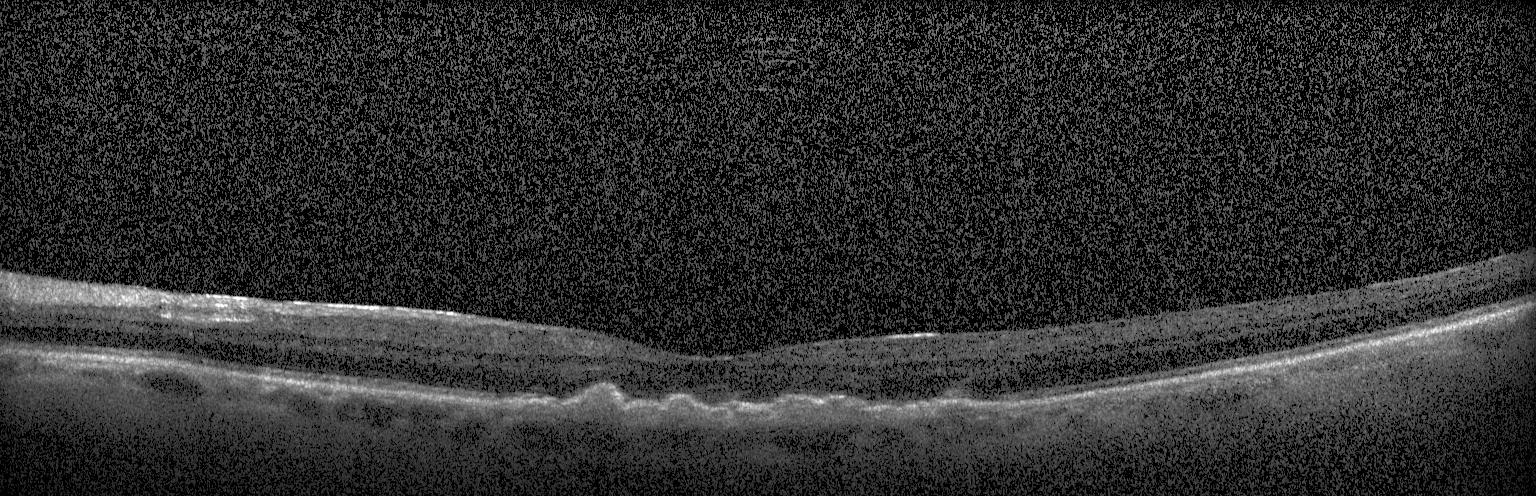

Multiple drusen.